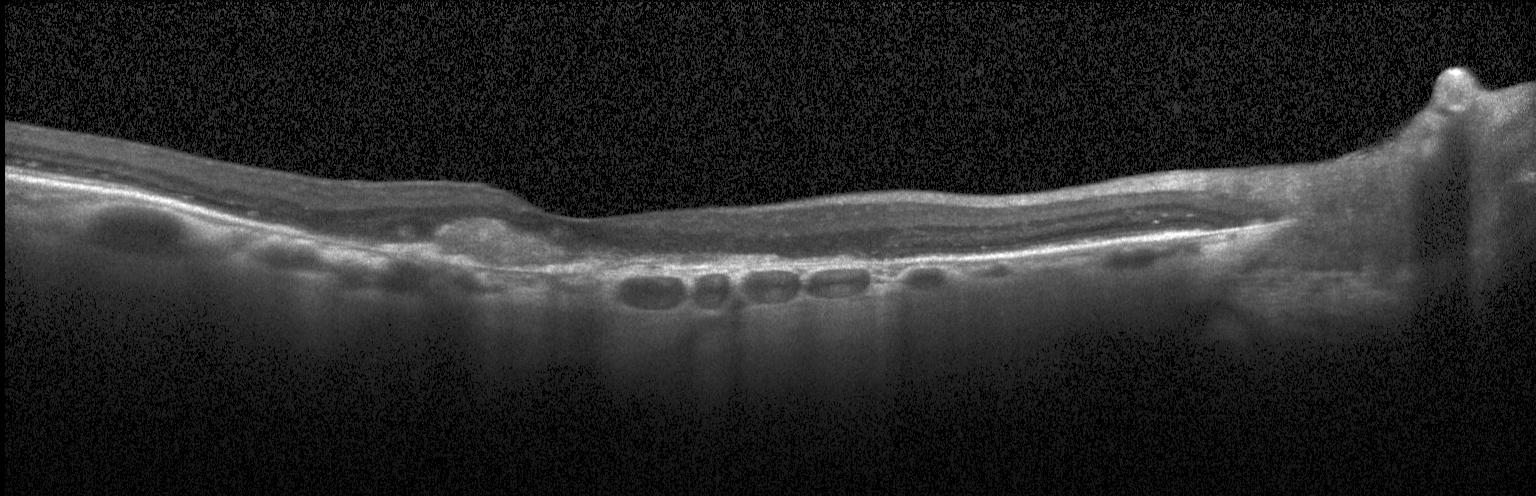 Impression: choroidal neovascularization (CNV).